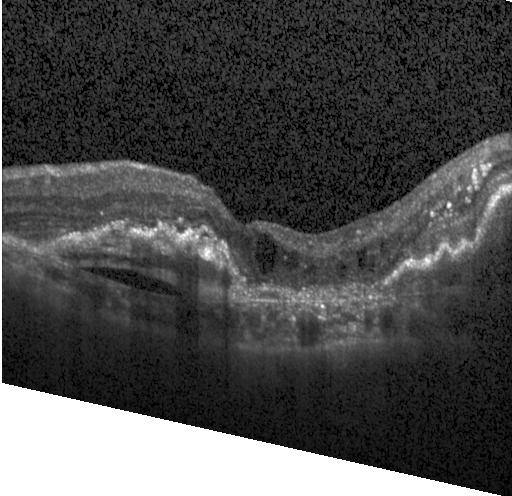
OCT line scan, macular scan — This B-scan demonstrates choroidal neovascularization.